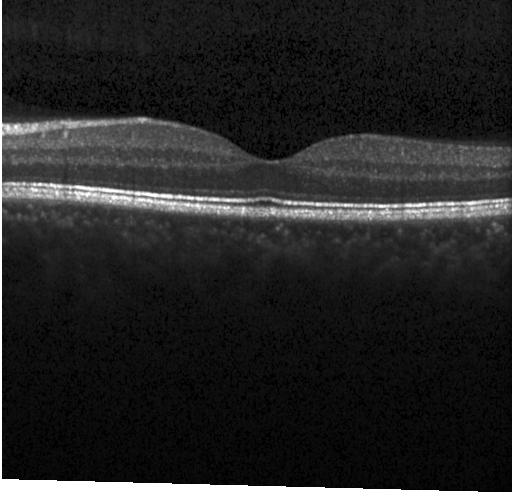 Dx: no choroidal neovascularization, diabetic macular edema, or drusen.